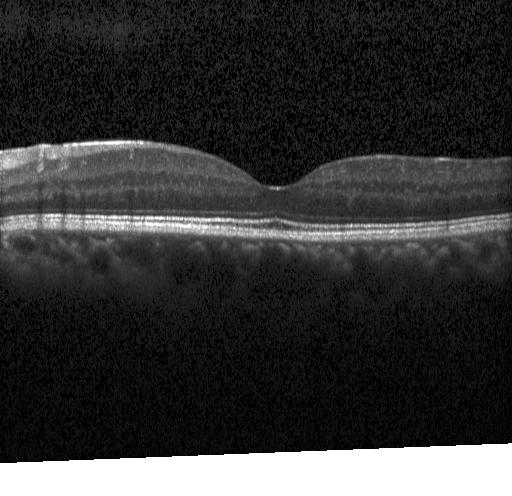
No choroidal neovascularization, no diabetic macular edema, and no drusen.